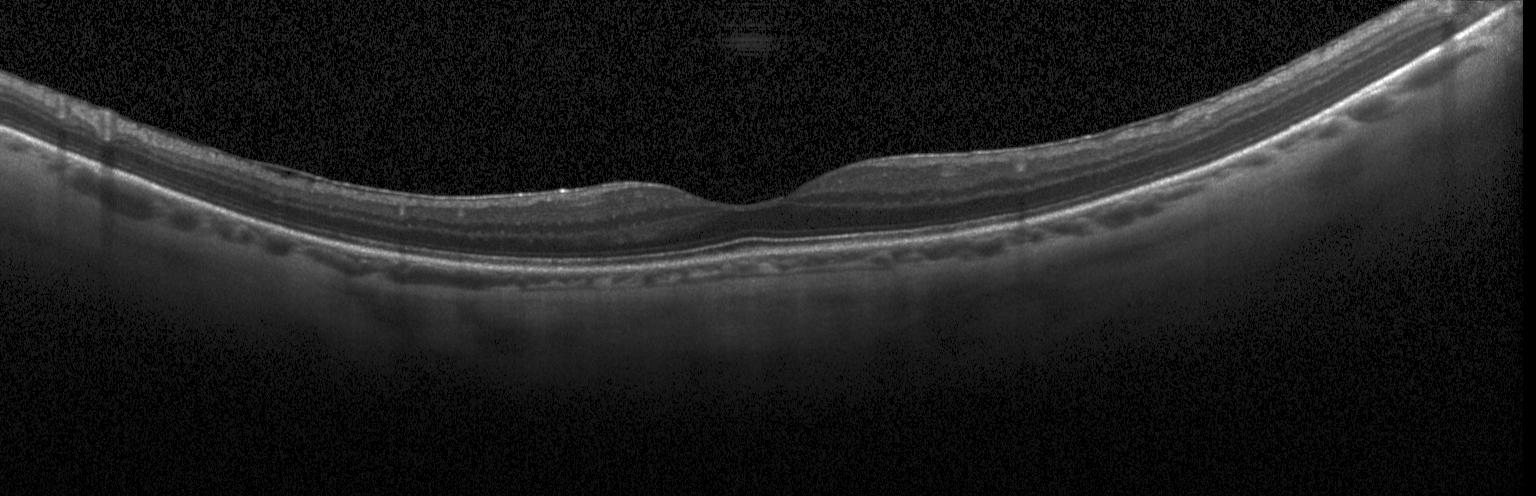

Optical coherence tomography B-scan, acquired on a Heidelberg Spectralis — Diagnosis: neither choroidal neovascularization, diabetic macular edema, nor drusen.